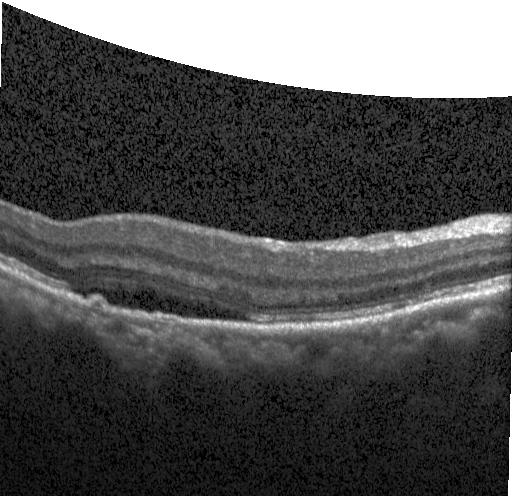

Optical coherence tomography B-scan · Heidelberg Spectralis OCT system · fovea-centered. Finding: a choroidal neovascular membrane.